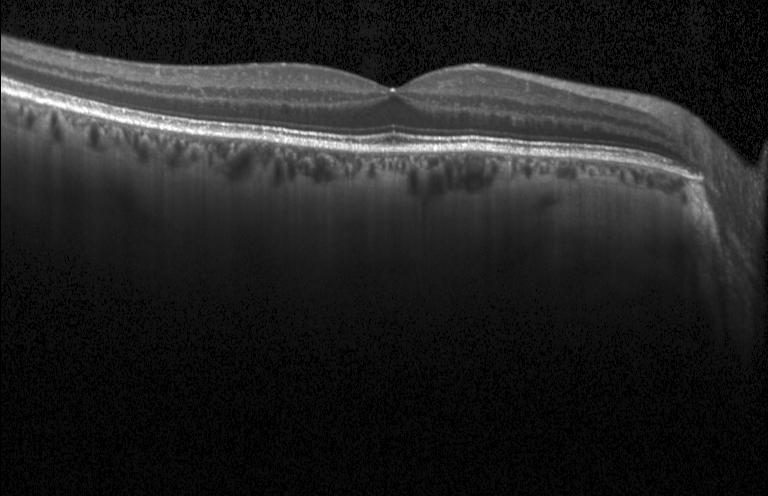

Diagnosis: no choroidal neovascularization, diabetic macular edema, or drusen.